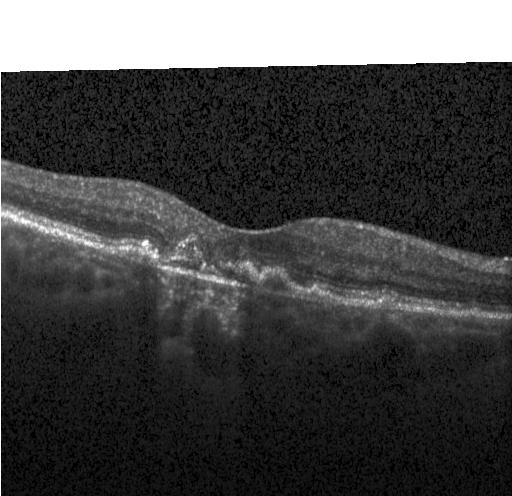 A choroidal neovascular membrane.